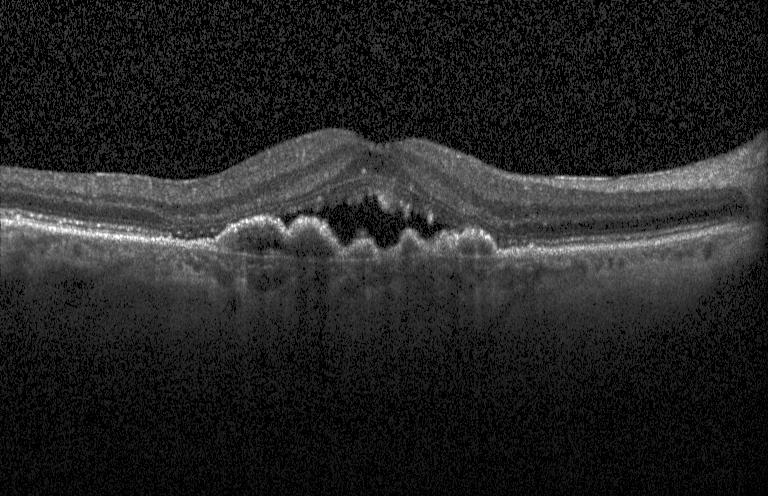

OCT line scan
This B-scan demonstrates choroidal neovascularization (CNV).